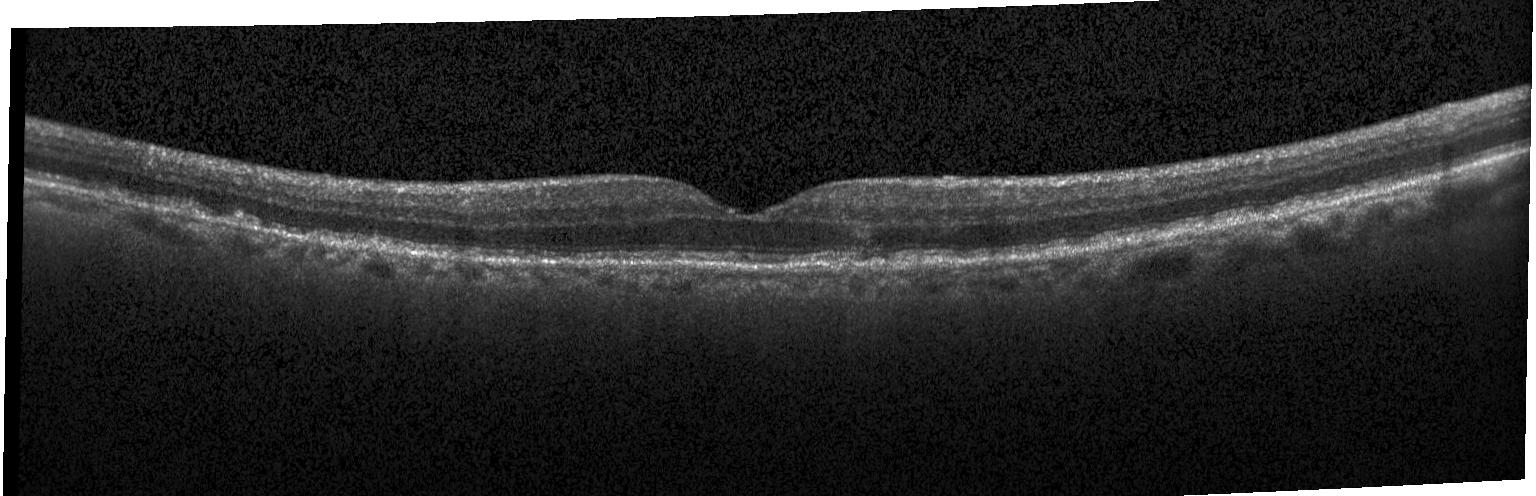

Centered on the fovea; spectral-domain optical coherence tomography; retinal OCT B-scan; Heidelberg Spectralis.
Assessment: drusen.